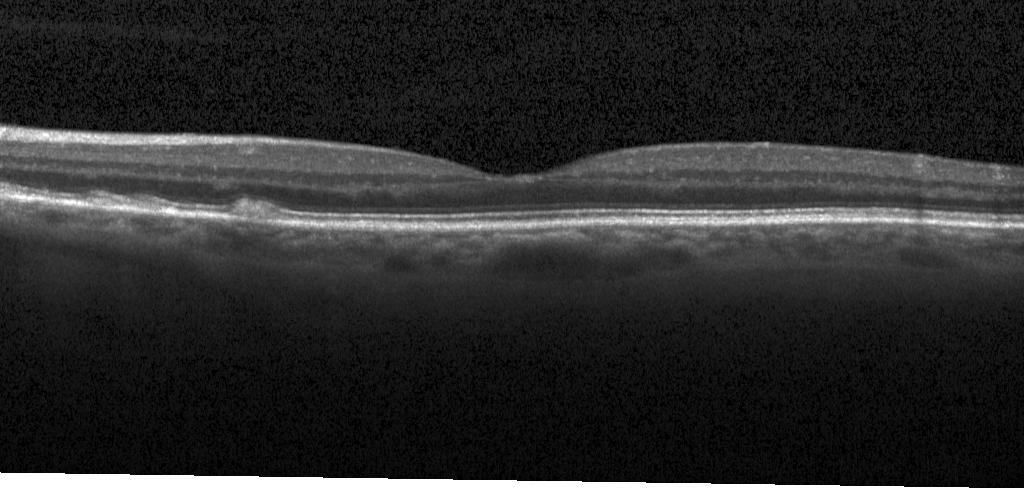
OCT B-scan showing multiple drusen.